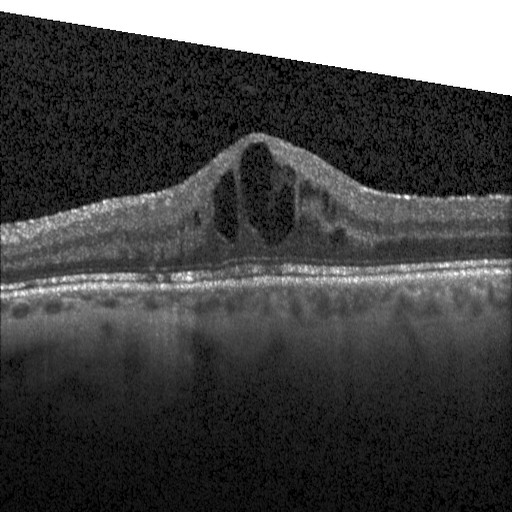

Spectral-domain OCT; retinal OCT B-scan; Heidelberg Spectralis; horizontal scan through the fovea
Finding: DME.